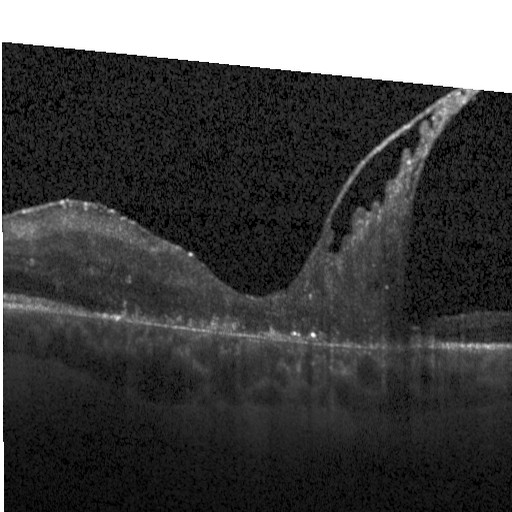 Macular scan · OCT B-scan · instrument: Heidelberg Spectralis · spectral-domain OCT — Macular OCT: DME.